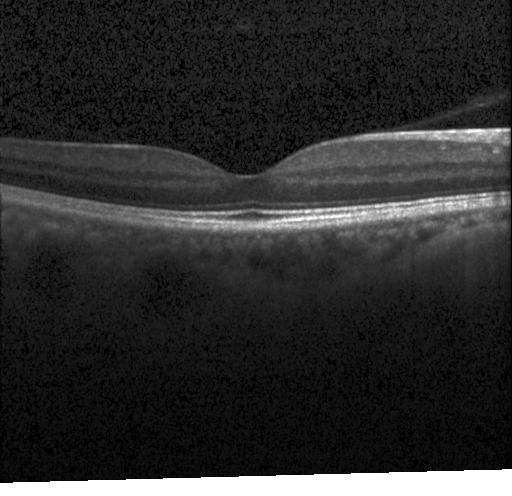

Macular scan. OCT B-scan.
Assessment: no CNV, no DME, and no drusen.